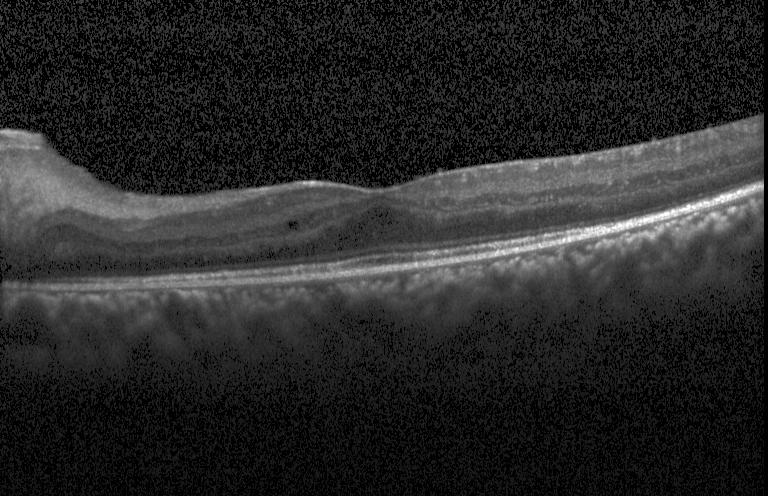

Instrument: Heidelberg Spectralis · OCT line scan — Diabetic macular edema (DME).